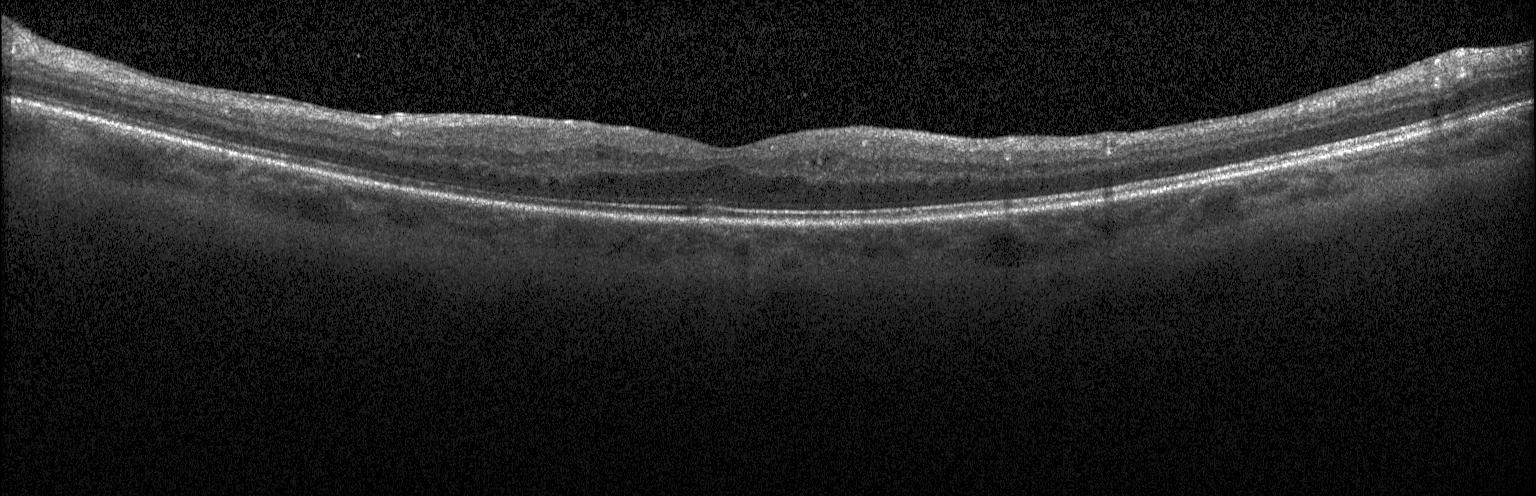
Instrument: Heidelberg Spectralis, retinal OCT B-scan, centered on the fovea. Assessment: DME.